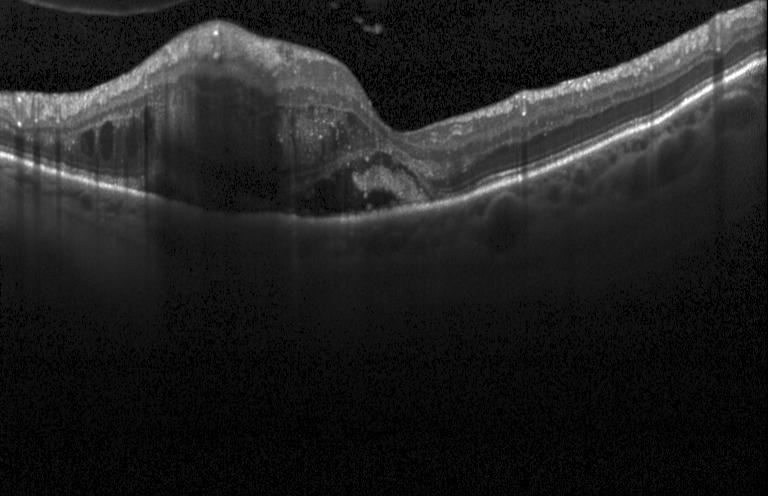
Retinal OCT cross-section · Heidelberg Spectralis OCT system · SD-OCT · through the macula
Impression: DME.